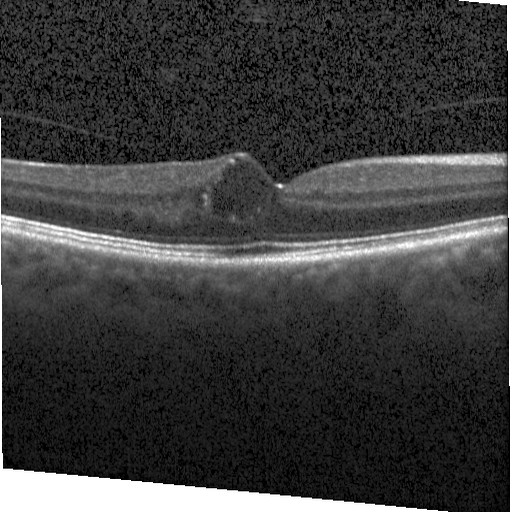 Retinal OCT B-scan — The scan shows diabetic macular edema (DME).